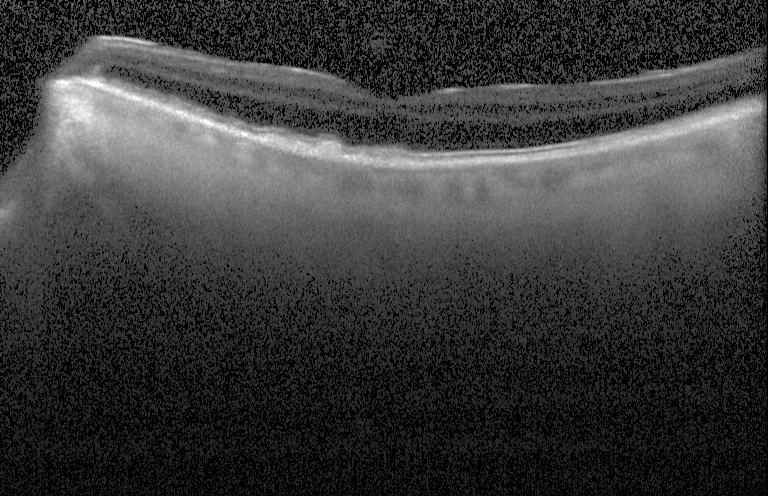
Retinal OCT B-scan · acquired on a Heidelberg Spectralis.
Diagnosis: multiple drusen.